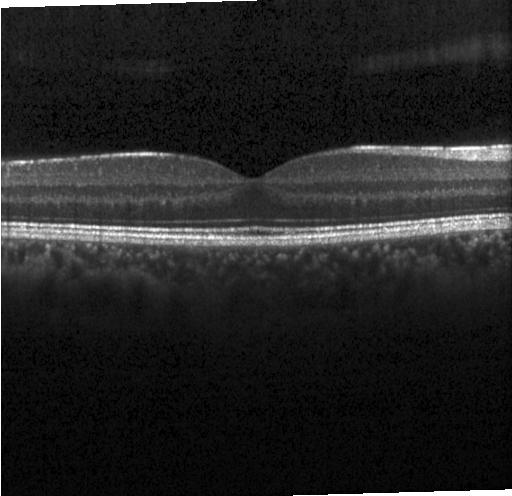
Retinal OCT B-scan; centered on the fovea
Finding: no CNV, DME, or drusen.